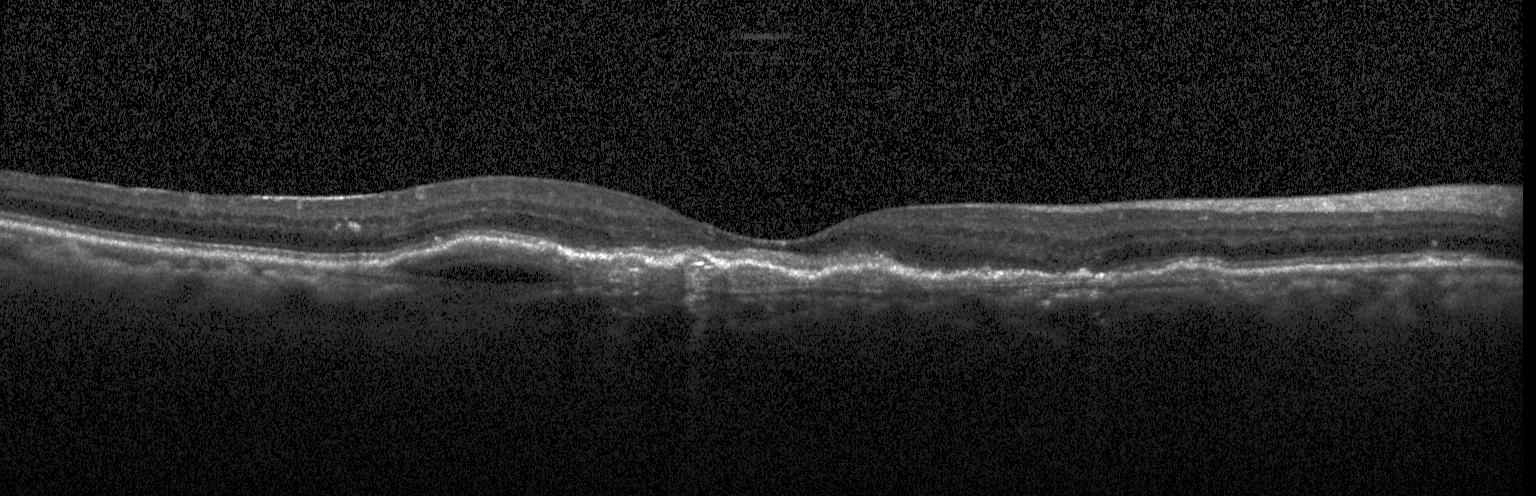 OCT finding: a choroidal neovascular membrane.